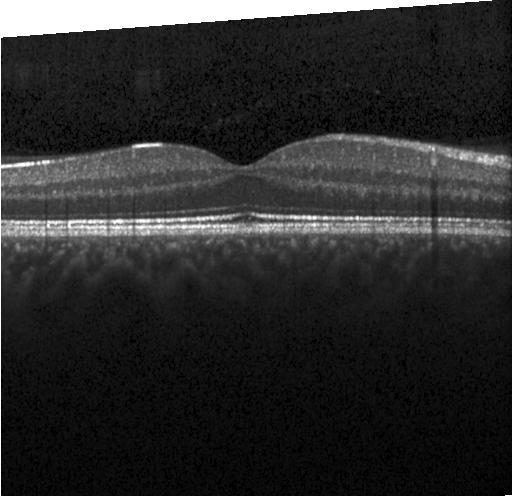 Acquired on a Heidelberg Spectralis · SD-OCT · fovea-centered · optical coherence tomography B-scan. Finding: no choroidal neovascularization, no diabetic macular edema, and no drusen.